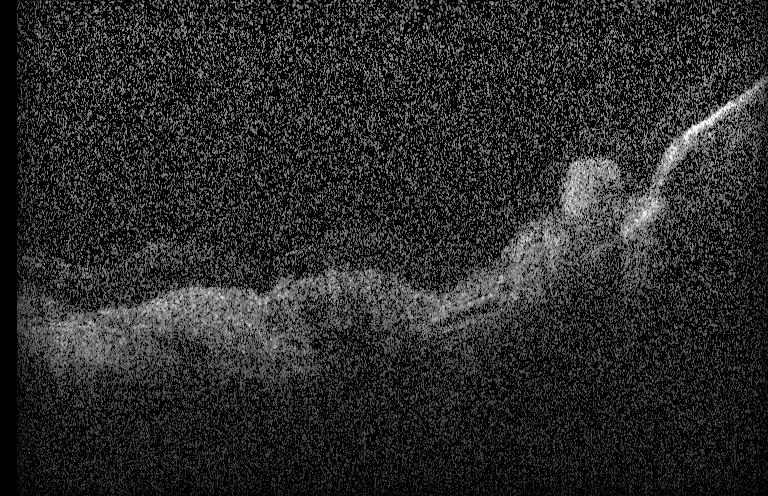

Finding: a choroidal neovascular membrane.